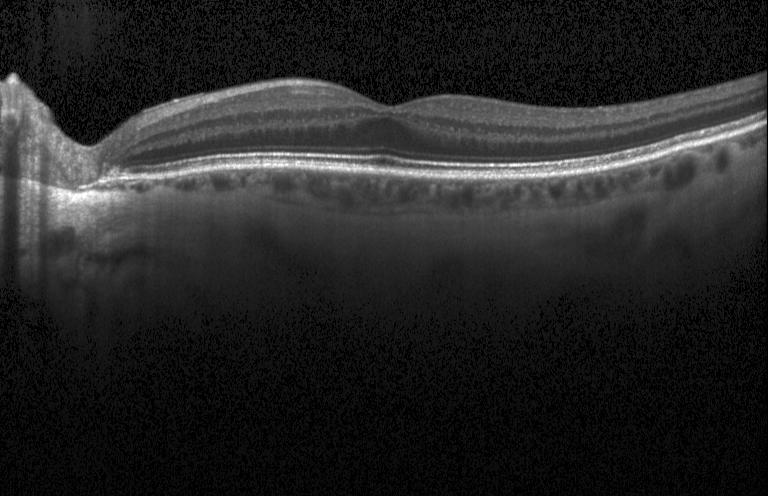
Heidelberg Spectralis OCT system · optical coherence tomography B-scan · through the macula.
No choroidal neovascularization, diabetic macular edema, or drusen.